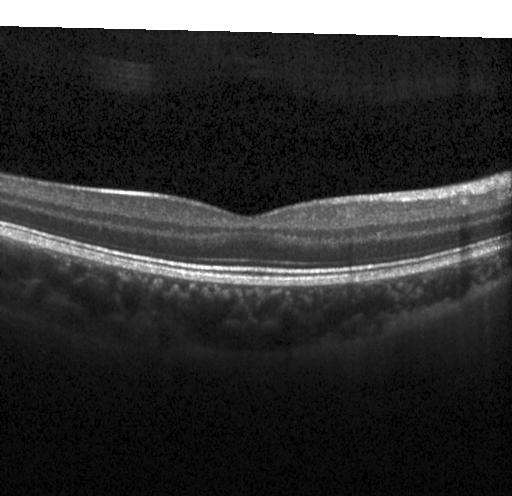

Impression: neither CNV, DME, nor drusen.